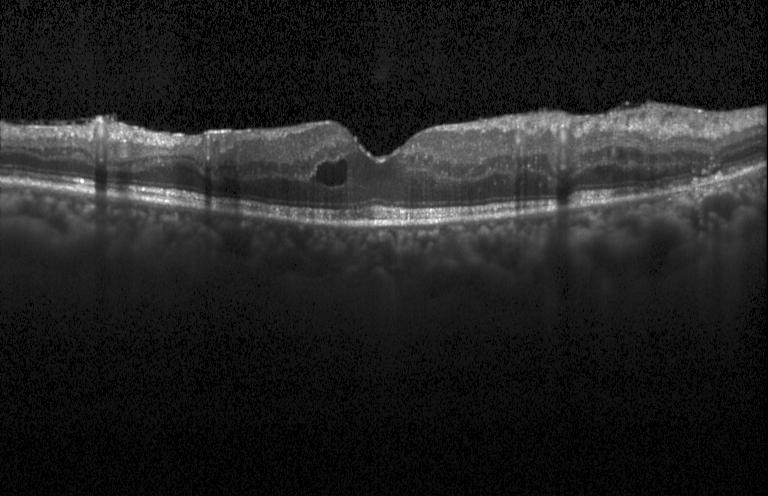

DME.